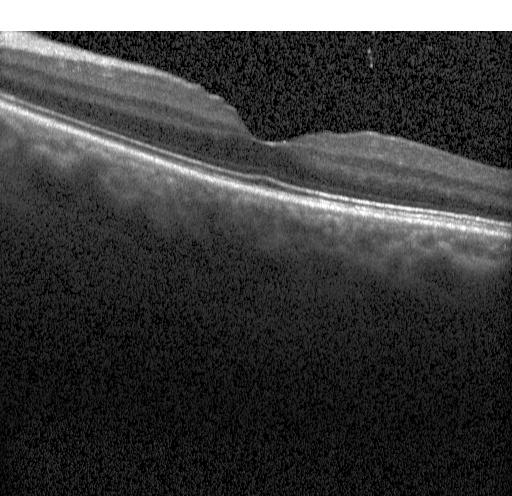

Fovea-centered; SD-OCT; Heidelberg Spectralis; OCT B-scan
Assessment: no choroidal neovascularization, diabetic macular edema, or drusen.